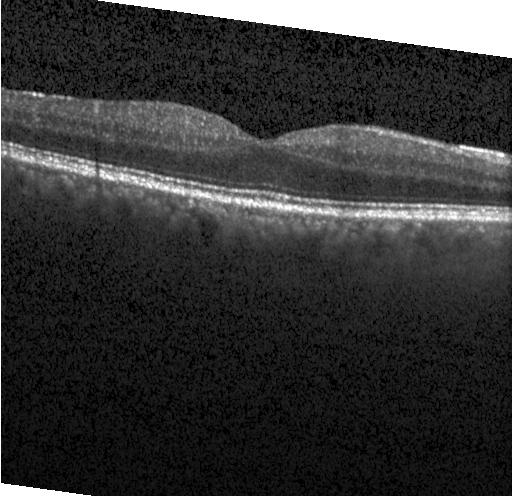 OCT line scan.
Dx: neither choroidal neovascularization, diabetic macular edema, nor drusen.